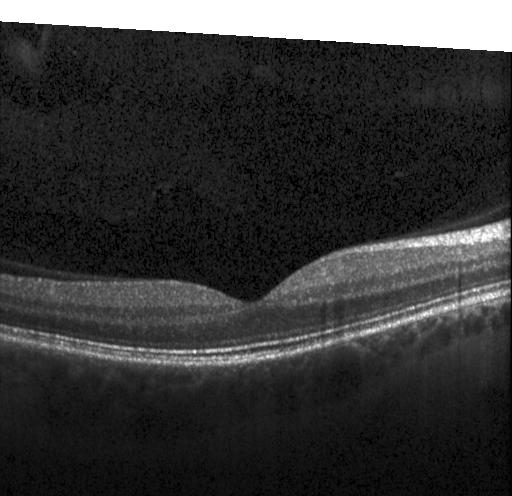 Fovea-centered, spectral-domain OCT, Heidelberg Spectralis, OCT B-scan. OCT finding: no CNV, no DME, and no drusen.